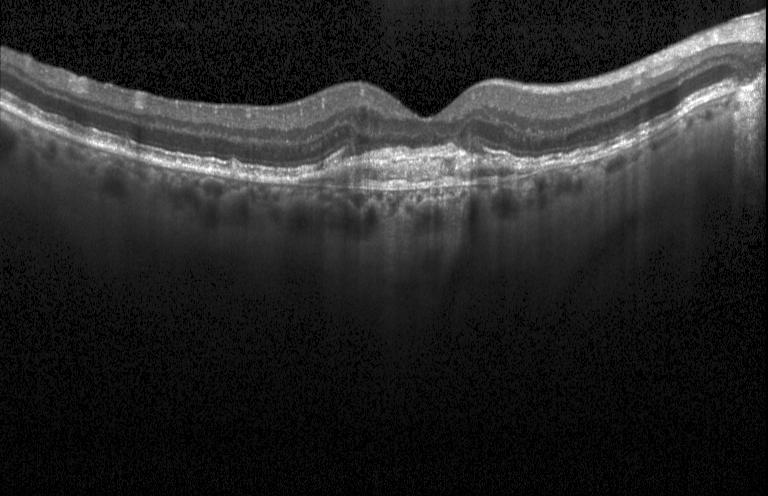

Spectral-domain OCT B-scan: a choroidal neovascular membrane.